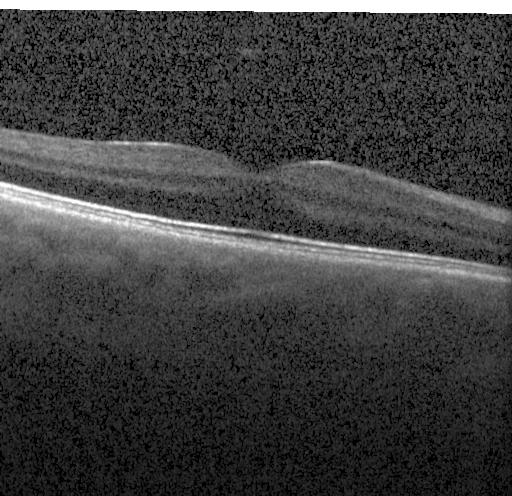

Impression: no evidence of choroidal neovascularization, diabetic macular edema, or drusen.